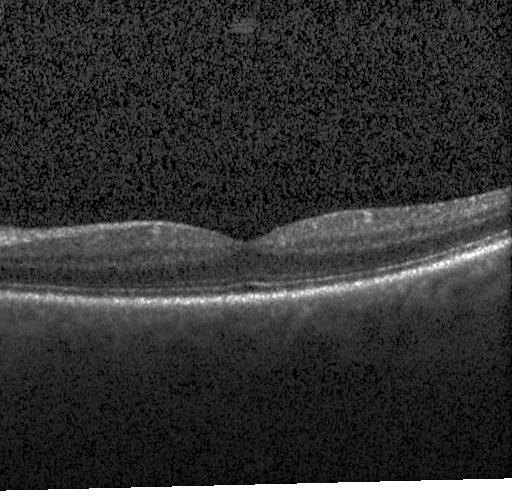
Finding: neither choroidal neovascularization, diabetic macular edema, nor drusen.